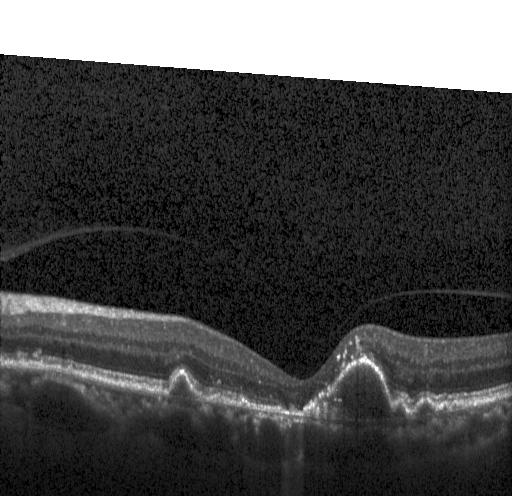
Choroidal neovascularization.